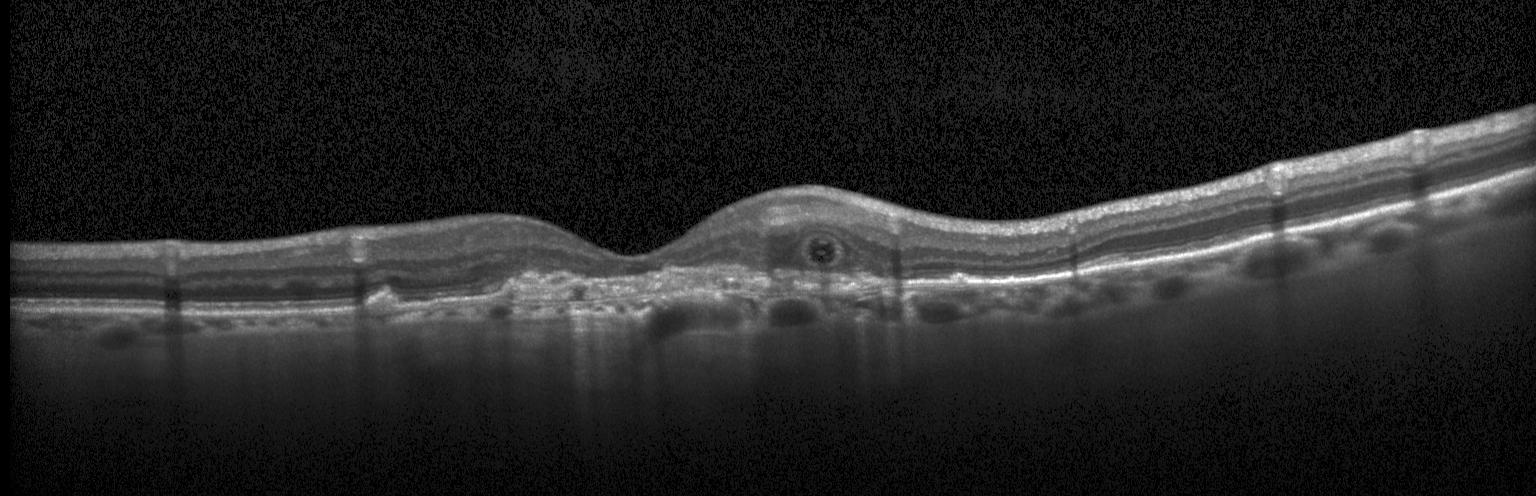
Acquired on a Heidelberg Spectralis; fovea-centered; spectral-domain optical coherence tomography; retinal OCT cross-section.
OCT finding: a choroidal neovascular membrane.